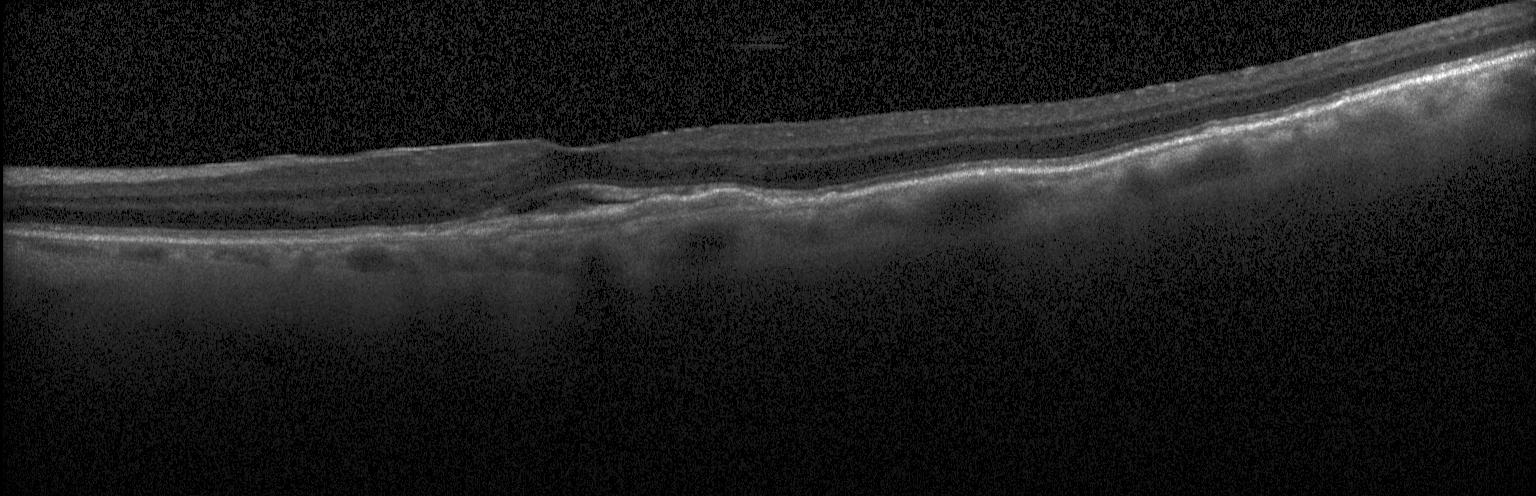

A choroidal neovascular membrane.